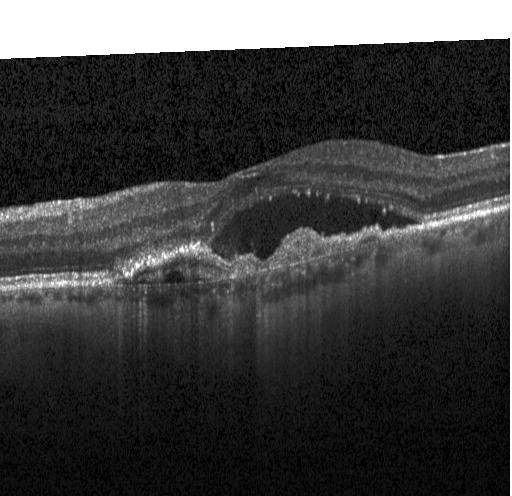
Optical coherence tomography scan
Assessment: choroidal neovascularization (CNV).